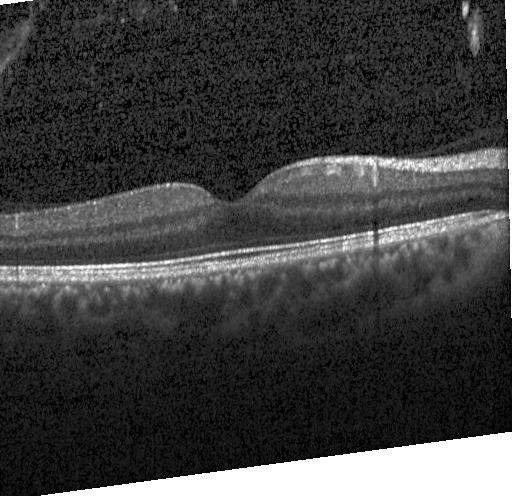 Retinal OCT cross-section · Heidelberg Spectralis OCT system · horizontal scan through the fovea.
Impression: no choroidal neovascularization, diabetic macular edema, or drusen.